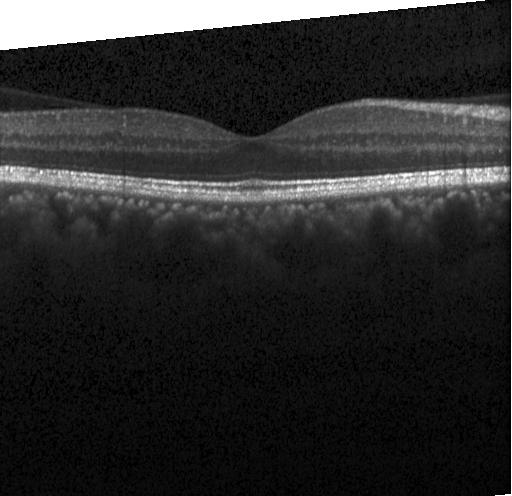 Heidelberg Spectralis OCT system; optical coherence tomography scan; fovea-centered
Impression: no CNV, no DME, and no drusen.